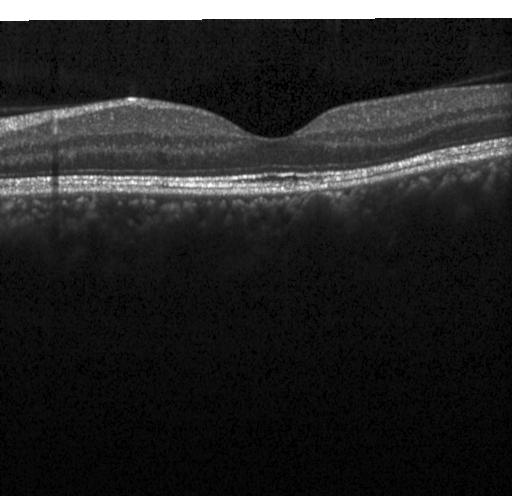 Instrument: Heidelberg Spectralis · spectral-domain OCT · OCT line scan — Impression: no evidence of CNV, DME, or drusen.